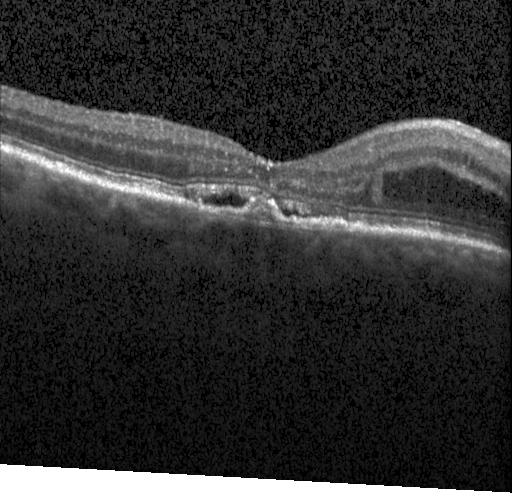 Centered on the fovea, Heidelberg Spectralis OCT system, spectral-domain optical coherence tomography, optical coherence tomography scan. This B-scan demonstrates CNV.